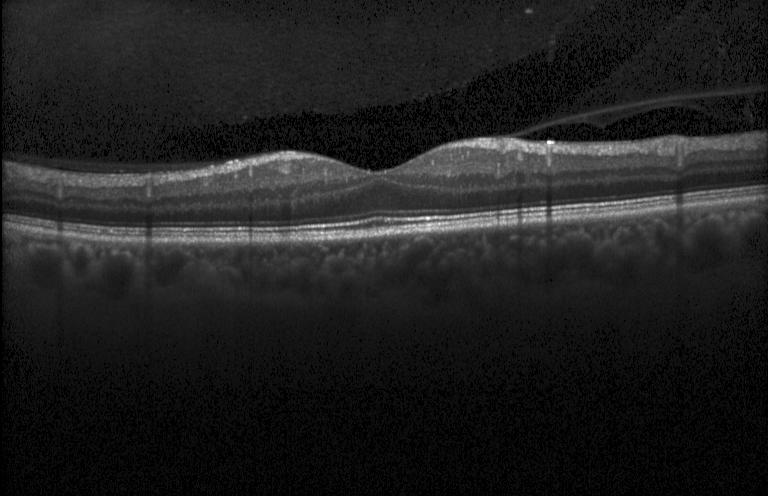

Heidelberg Spectralis; optical coherence tomography B-scan. Impression: no evidence of CNV, DME, or drusen.